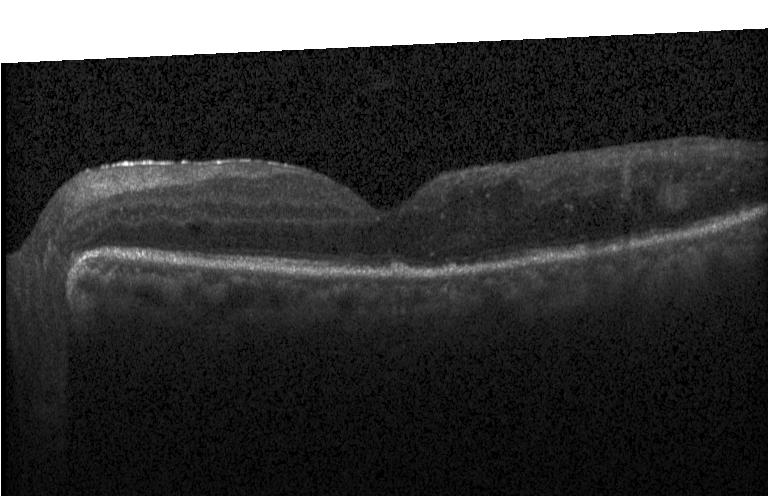

Diagnosis: DME.